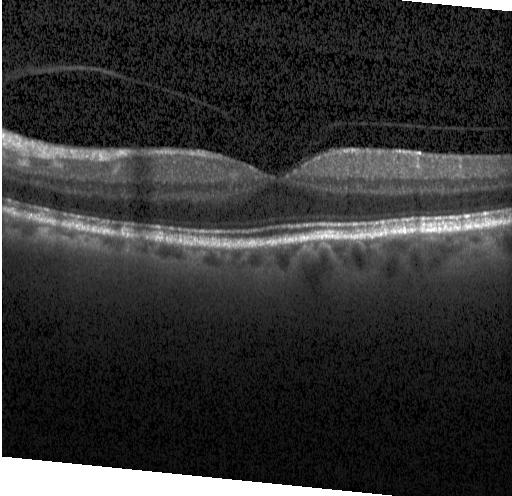
Diagnosis: no choroidal neovascularization, no diabetic macular edema, and no drusen.